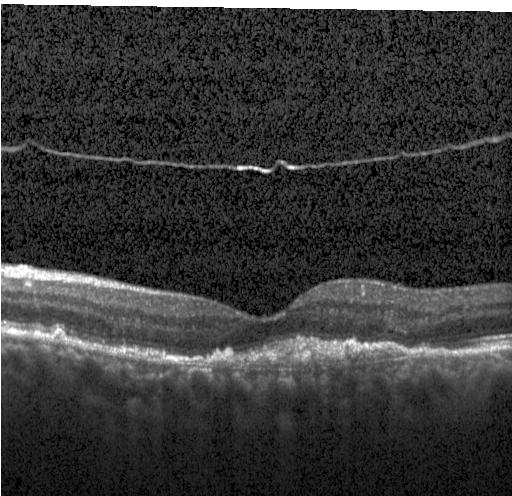

Spectral-domain OCT B-scan: a choroidal neovascular membrane.